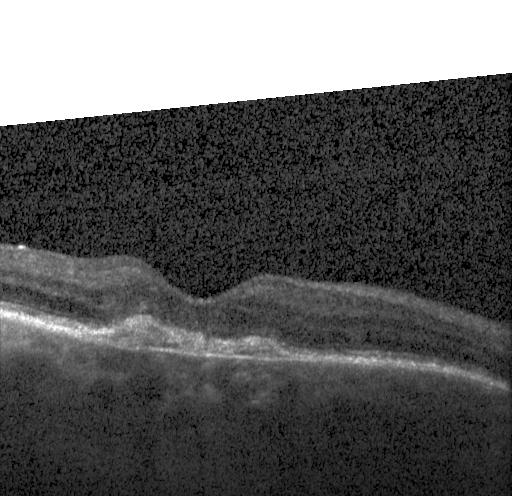 Retinal OCT B-scan
A choroidal neovascular membrane.